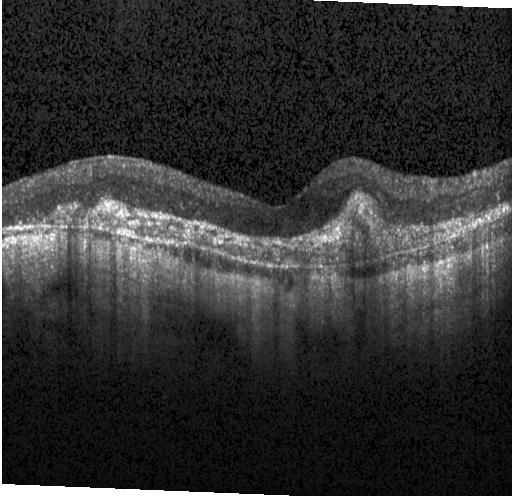

Retinal OCT cross-section showing a choroidal neovascular membrane.